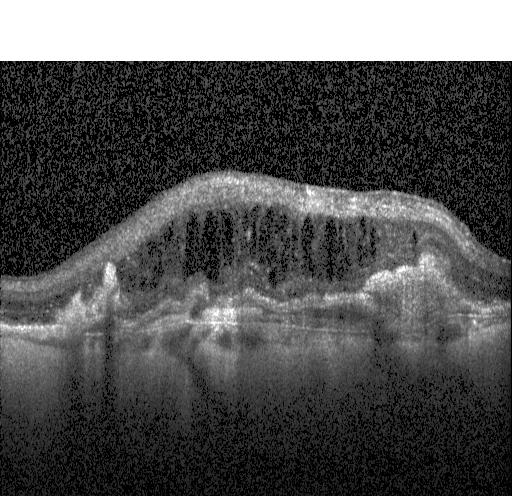 Optical coherence tomography scan. Instrument: Heidelberg Spectralis.
Diagnosis: a choroidal neovascular membrane.